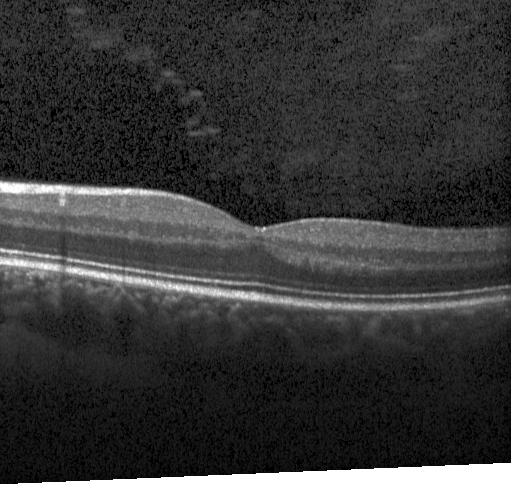
Heidelberg Spectralis OCT system; SD-OCT; OCT B-scan; centered on the fovea — No choroidal neovascularization, no diabetic macular edema, and no drusen.